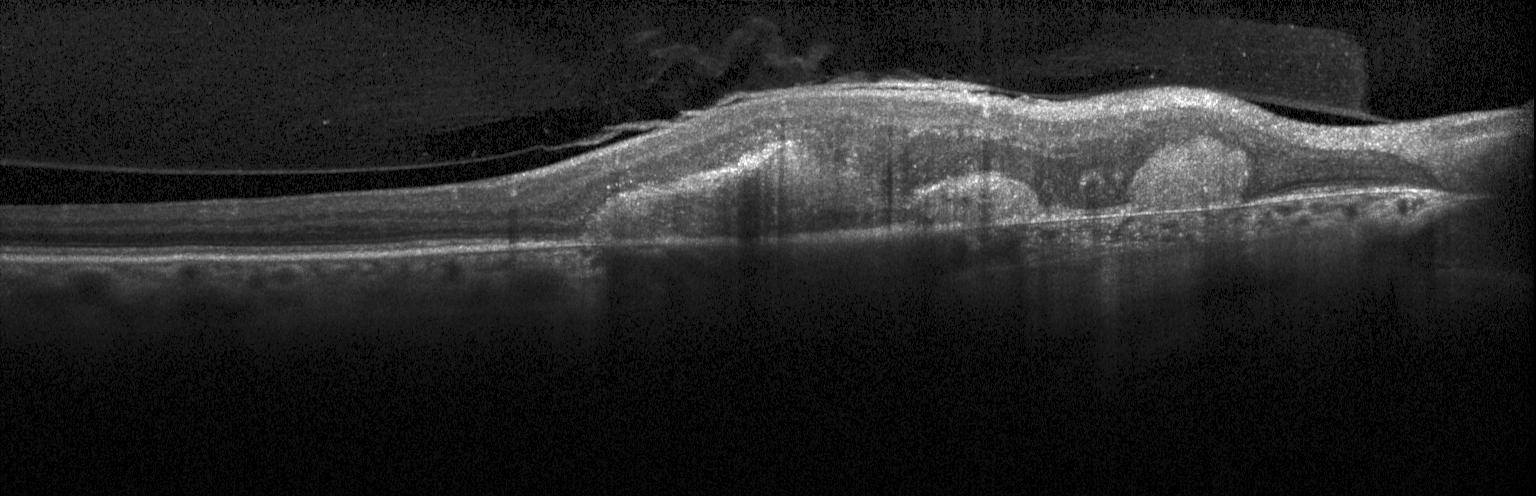
Optical coherence tomography scan; horizontal scan through the fovea. This B-scan demonstrates a choroidal neovascular membrane.